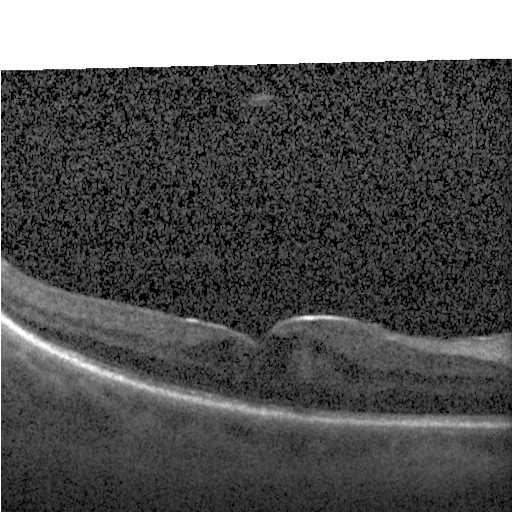 Assessment: diabetic macular edema (DME).